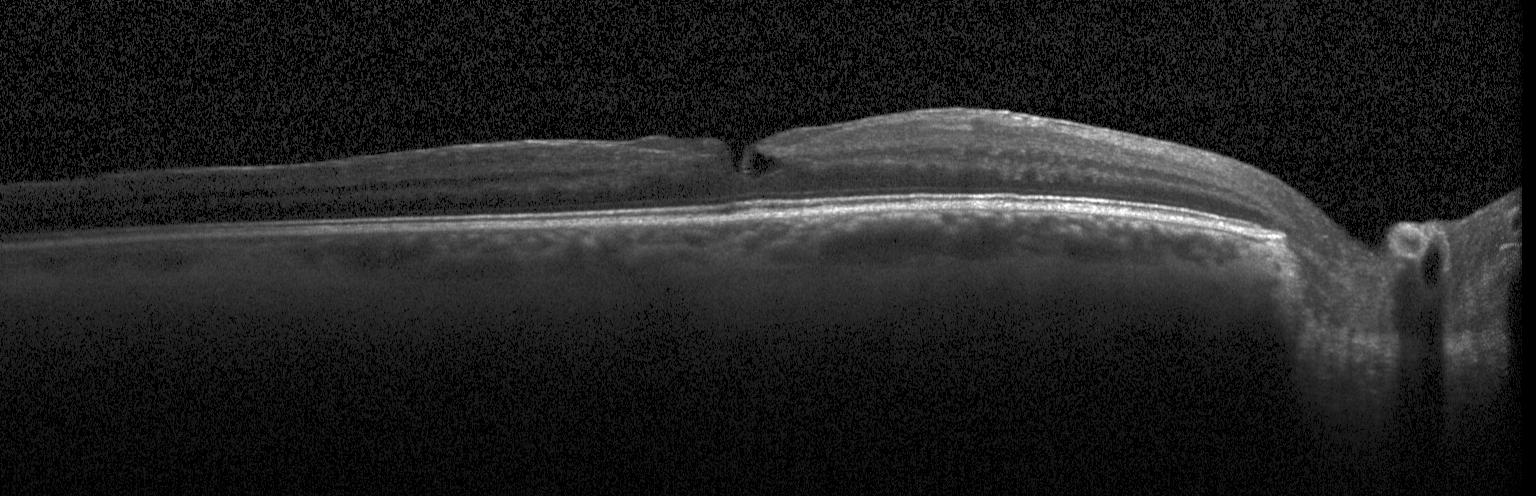 Heidelberg Spectralis; horizontal scan through the fovea; SD-OCT; optical coherence tomography scan — Assessment: diabetic macular edema.